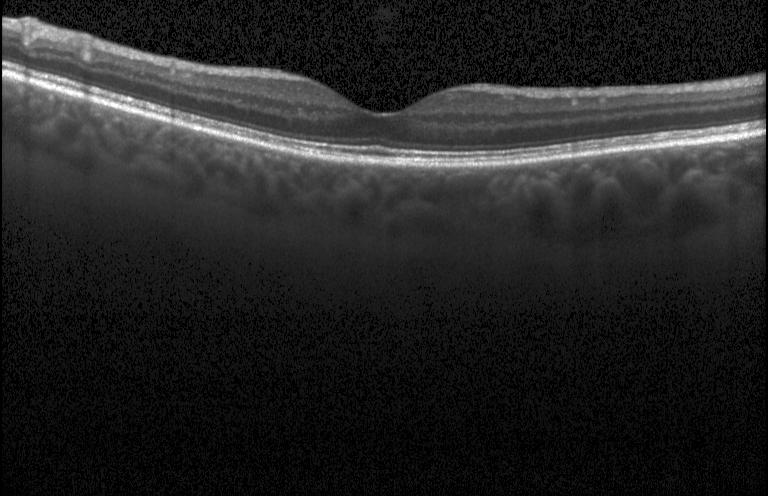

Fovea-centered; OCT line scan; SD-OCT
Finding: no choroidal neovascularization, diabetic macular edema, or drusen.